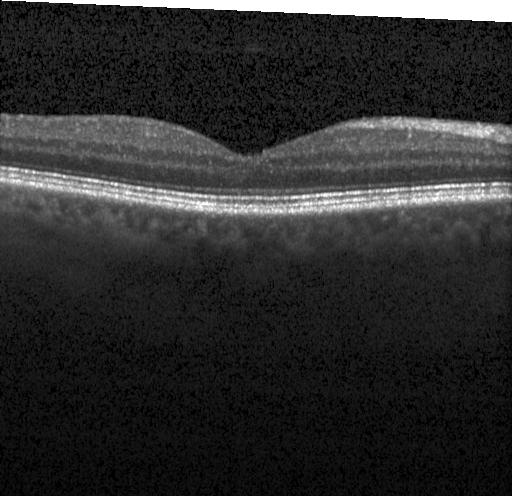
Impression: no evidence of choroidal neovascularization, diabetic macular edema, or drusen.